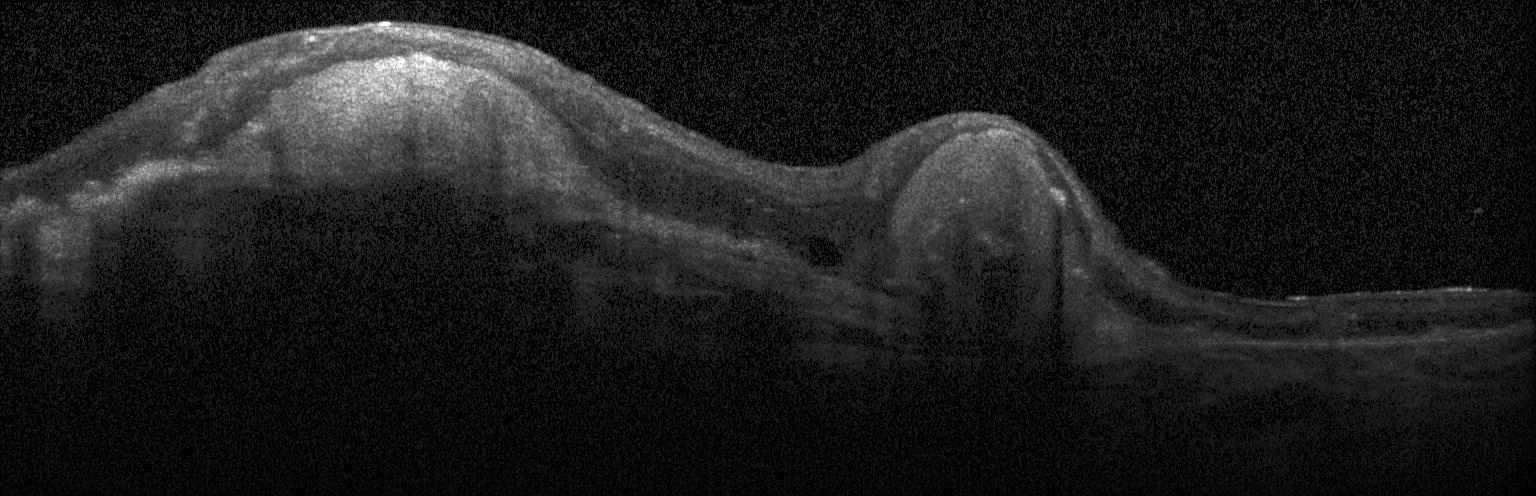
OCT finding: a choroidal neovascular membrane.